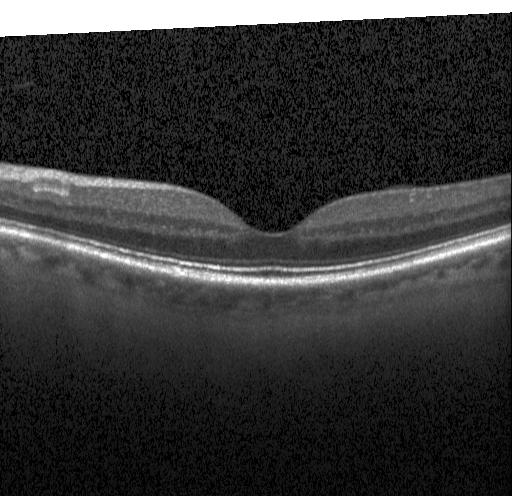
Dx: neither choroidal neovascularization, diabetic macular edema, nor drusen.